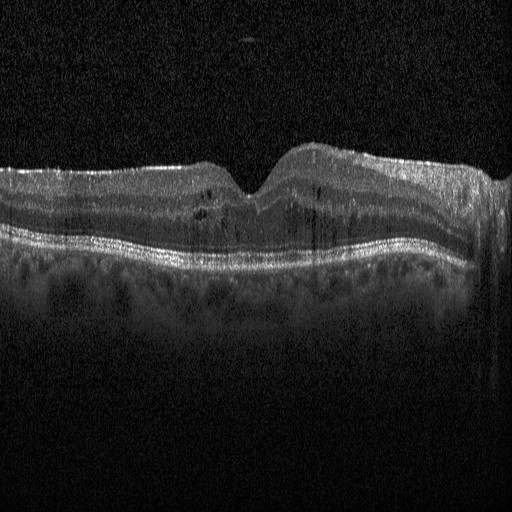
Heidelberg Spectralis. Fovea-centered. Optical coherence tomography scan
This B-scan demonstrates diabetic macular edema (DME).